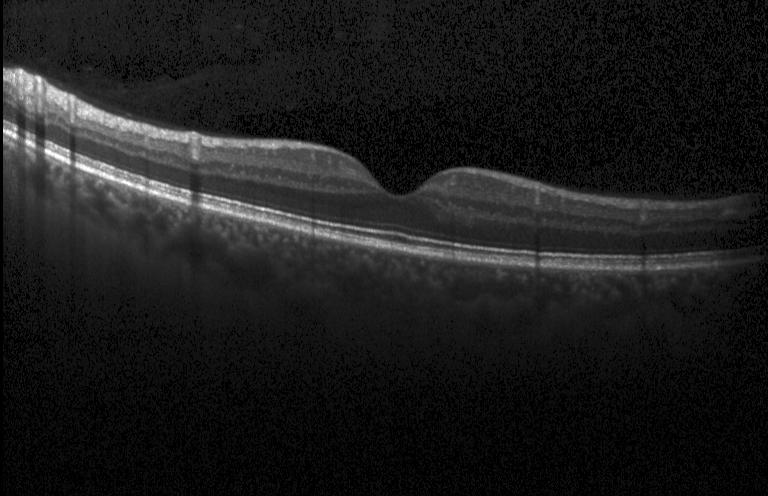

Macular scan, retinal OCT cross-section
OCT finding: no choroidal neovascularization, diabetic macular edema, or drusen.